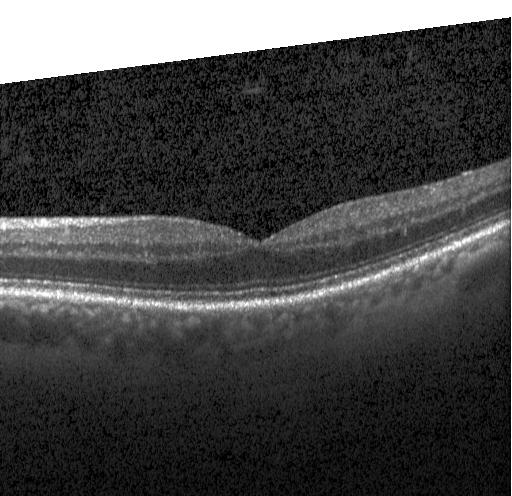
Heidelberg Spectralis OCT system; optical coherence tomography scan
Assessment: no evidence of choroidal neovascularization, diabetic macular edema, or drusen.